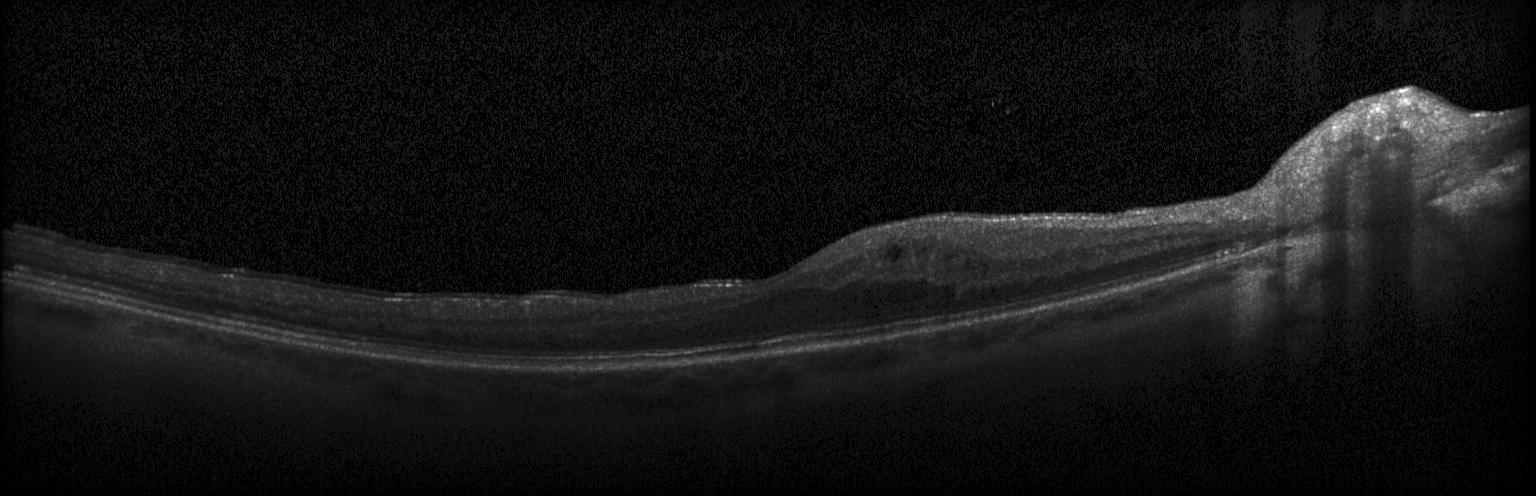

Heidelberg Spectralis OCT system; SD-OCT; retinal OCT cross-section; fovea-centered — Diabetic macular edema (DME).